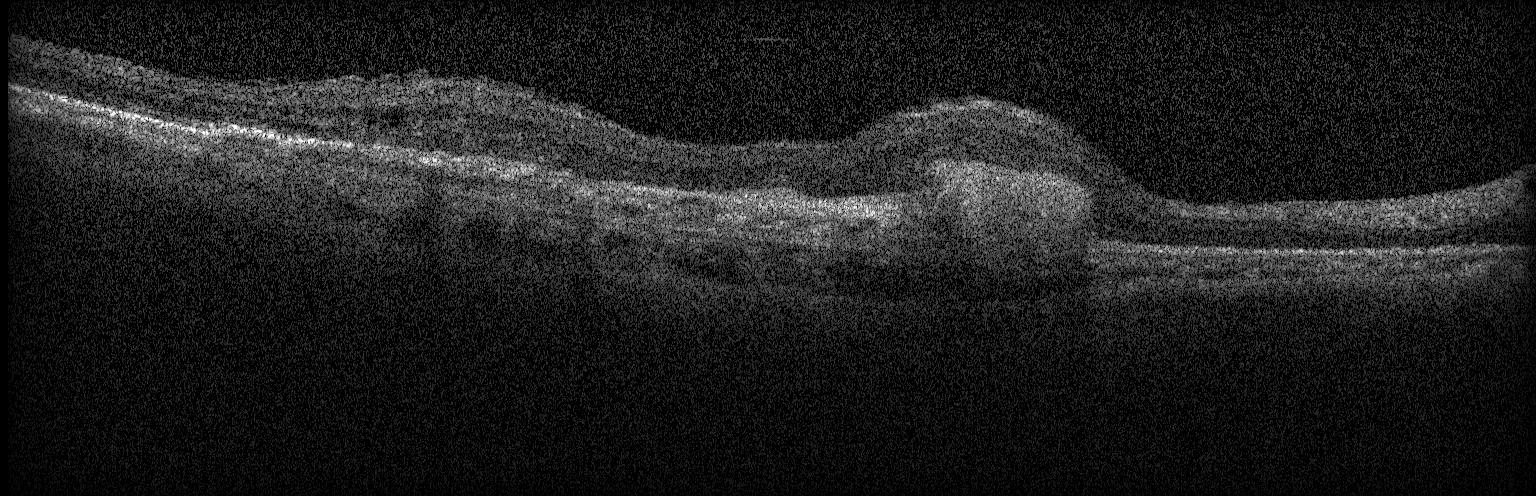

OCT B-scan · spectral-domain OCT — This B-scan demonstrates a choroidal neovascular membrane.